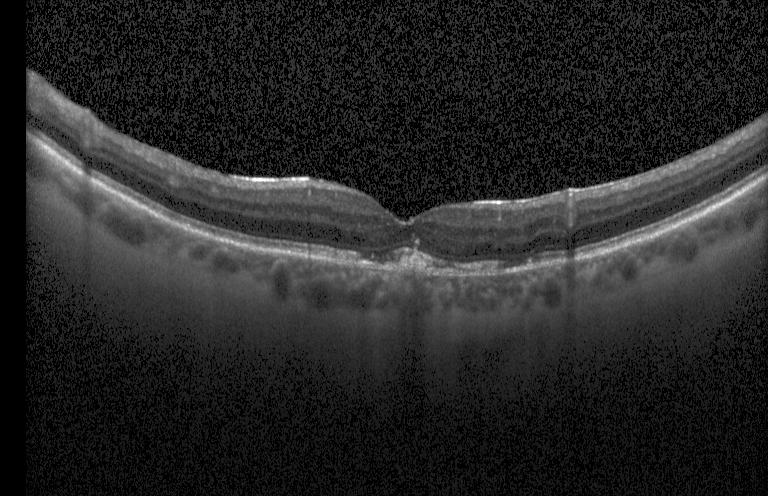 Optical coherence tomography scan; through the macula.
Finding: choroidal neovascularization.